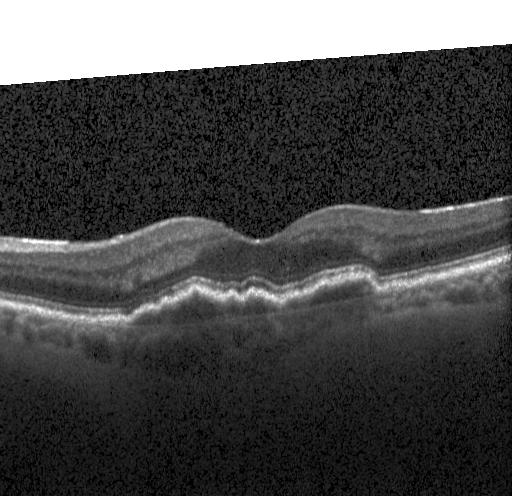

Retinal OCT cross-section. The scan shows choroidal neovascularization (CNV).